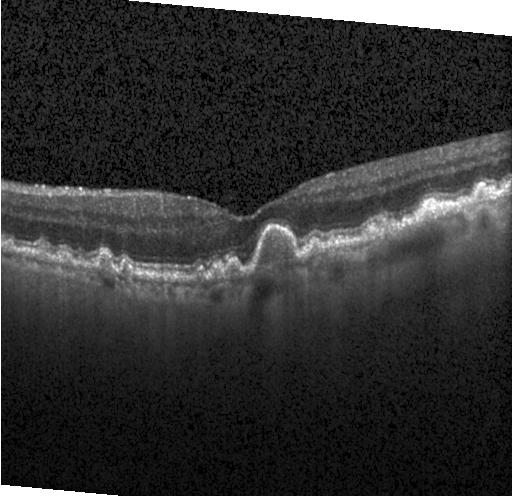
SD-OCT; instrument: Heidelberg Spectralis; retinal OCT B-scan; through the macula.
Finding: multiple drusen.